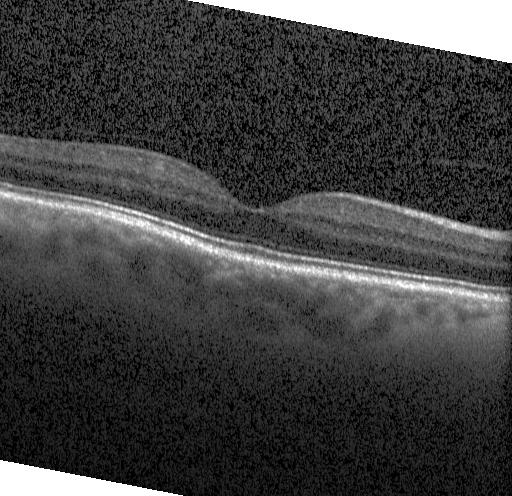 Acquired on a Heidelberg Spectralis, OCT B-scan, through the macula, spectral-domain OCT
Finding: neither CNV, DME, nor drusen.